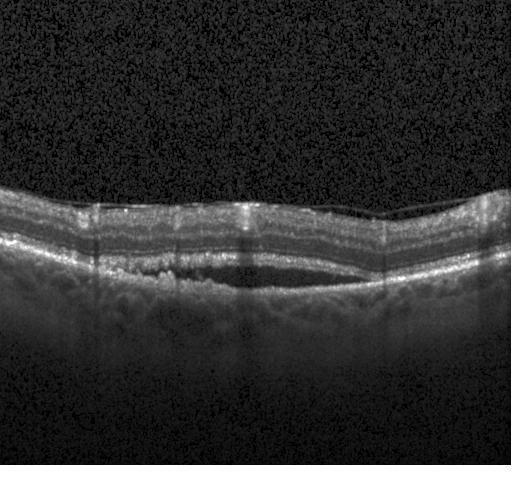
OCT finding: a choroidal neovascular membrane.